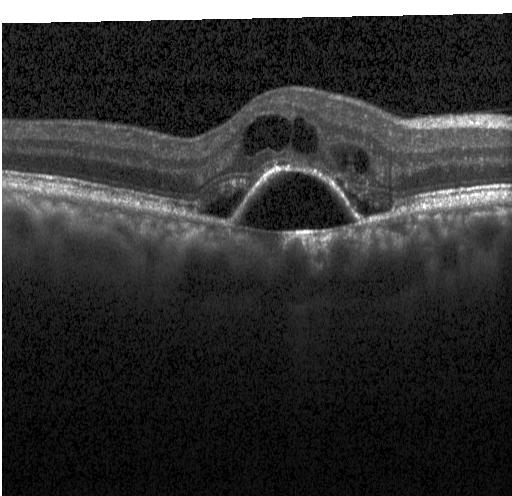 Retinal OCT cross-section
Finding: a choroidal neovascular membrane.